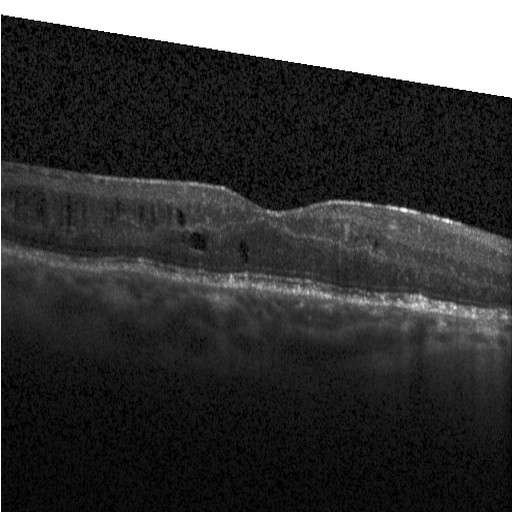

SD-OCT · OCT B-scan.
Finding: diabetic macular edema (DME).